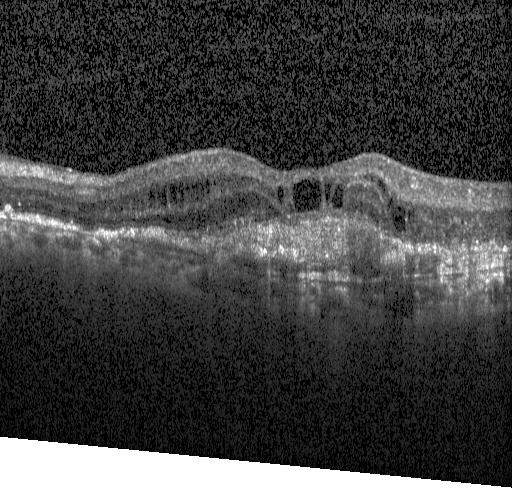

OCT finding: a choroidal neovascular membrane.